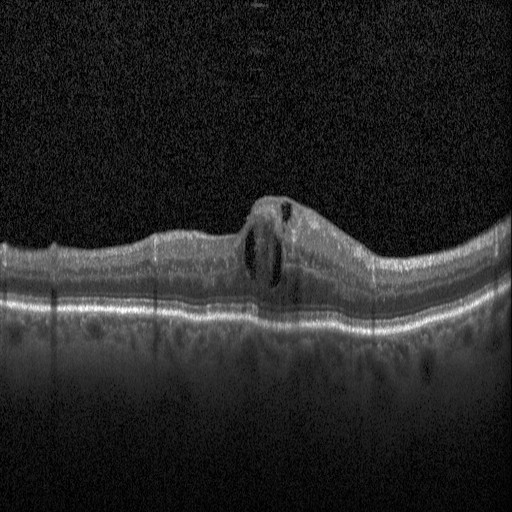 Impression: DME.